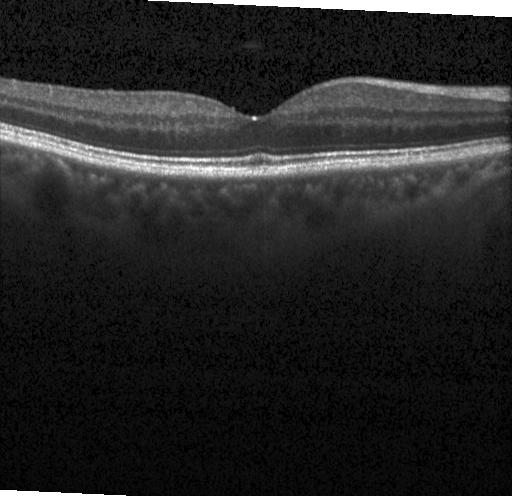 OCT line scan.
The scan shows no choroidal neovascularization, no diabetic macular edema, and no drusen.